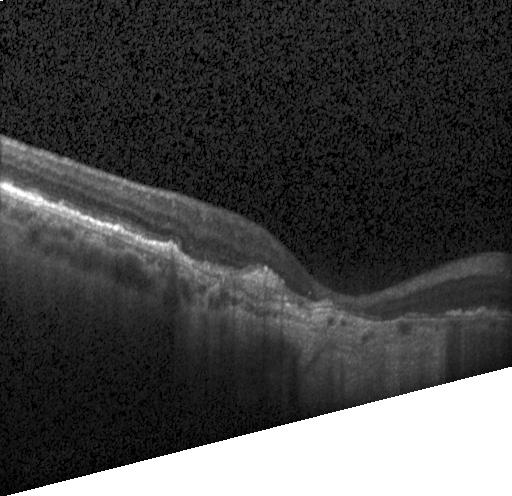 Macular scan; OCT B-scan; SD-OCT; Heidelberg Spectralis
The scan shows CNV.